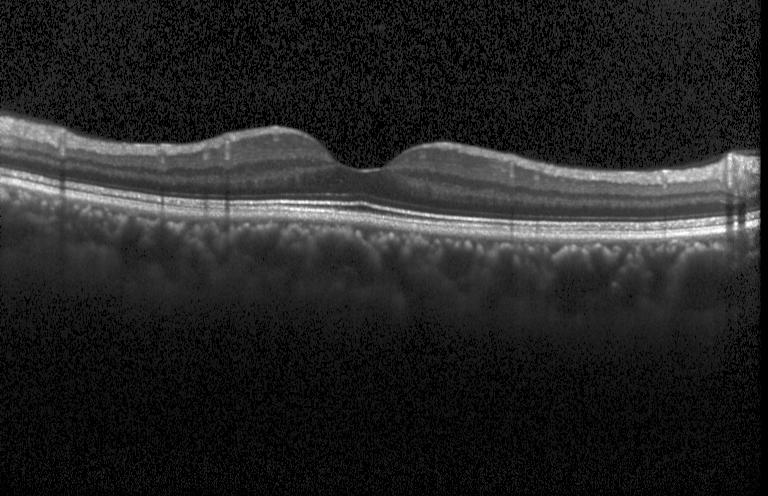
Spectral-domain optical coherence tomography · acquired on a Heidelberg Spectralis · retinal OCT cross-section
OCT finding: neither CNV, DME, nor drusen.